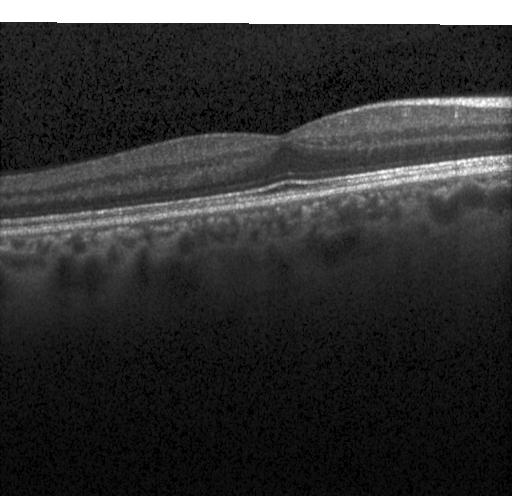 Finding: neither CNV, DME, nor drusen.